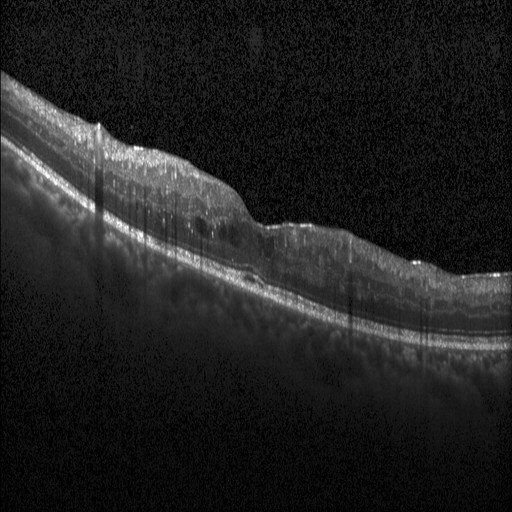
Optical coherence tomography B-scan; spectral-domain optical coherence tomography — The scan shows DME.